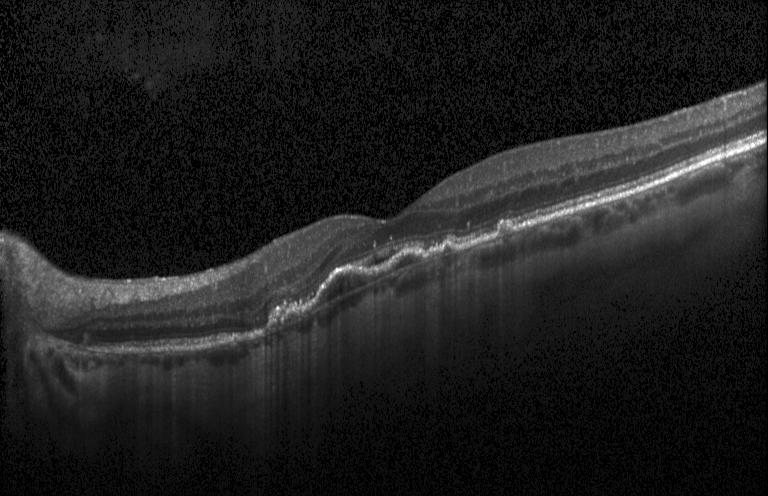 Optical coherence tomography B-scan. Assessment: choroidal neovascularization (CNV).